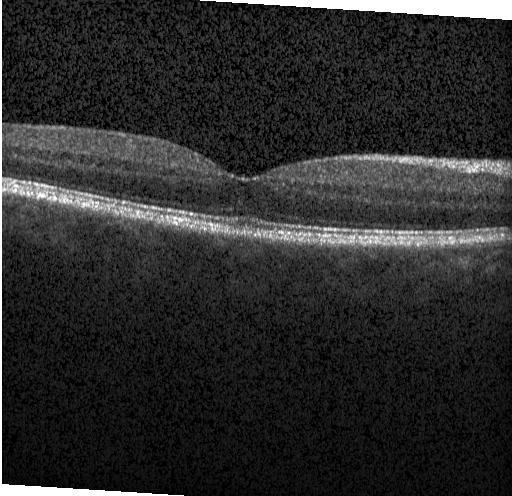 Retinal OCT B-scan, through the macula, spectral-domain OCT.
The scan shows neither choroidal neovascularization, diabetic macular edema, nor drusen.